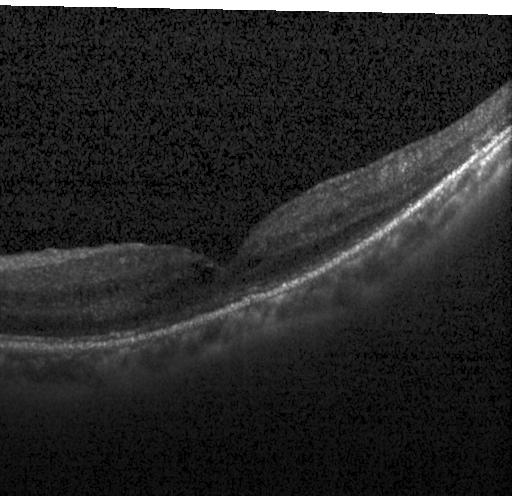 Retinal OCT cross-section. This B-scan demonstrates diabetic macular edema (DME).